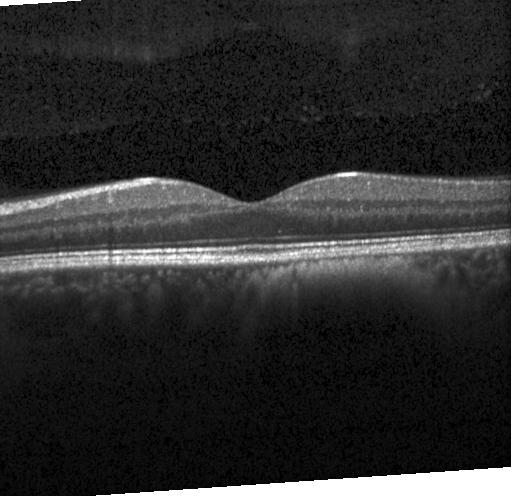 Retinal OCT cross-section. Heidelberg Spectralis OCT system. Spectral-domain optical coherence tomography. Diagnosis: no choroidal neovascularization, diabetic macular edema, or drusen.